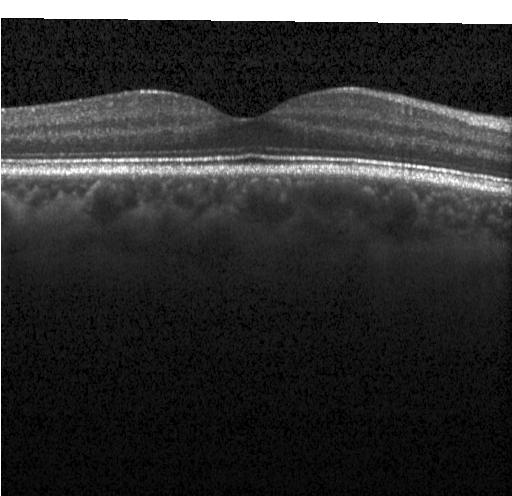

Optical coherence tomography B-scan; spectral-domain optical coherence tomography; fovea-centered; Heidelberg Spectralis. Impression: no evidence of CNV, DME, or drusen.